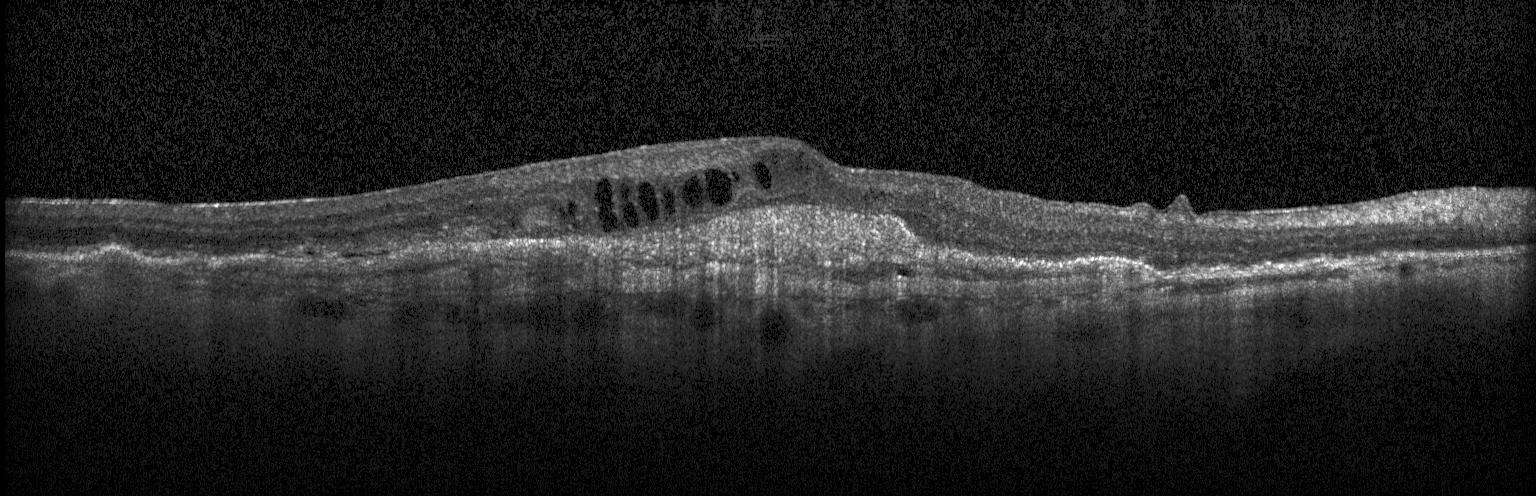

OCT line scan; SD-OCT.
This B-scan demonstrates CNV.